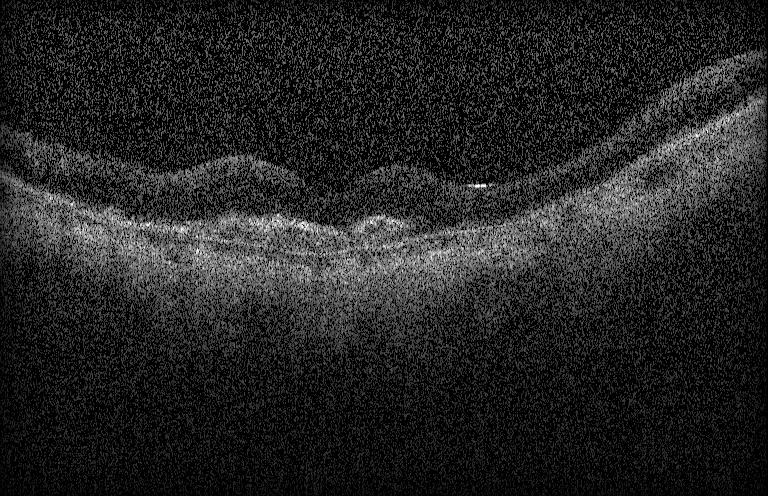

Retinal OCT B-scan, SD-OCT, Heidelberg Spectralis OCT system, horizontal scan through the fovea. Choroidal neovascularization.